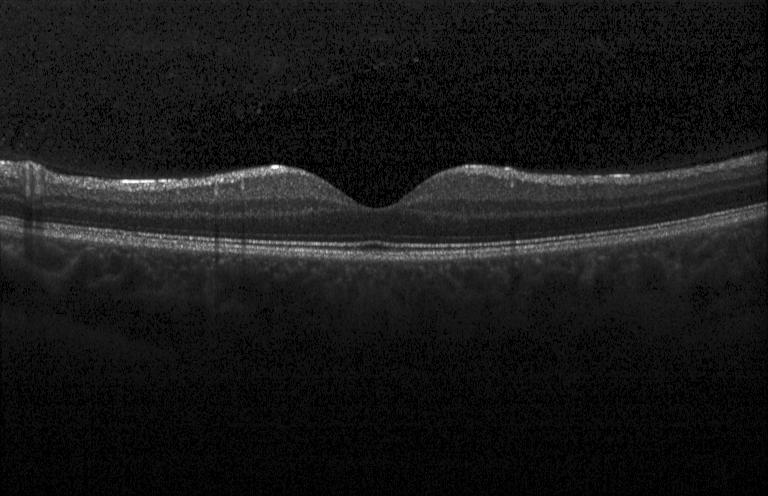 Fovea-centered; acquired on a Heidelberg Spectralis; OCT line scan — Macular OCT: no evidence of choroidal neovascularization, diabetic macular edema, or drusen.